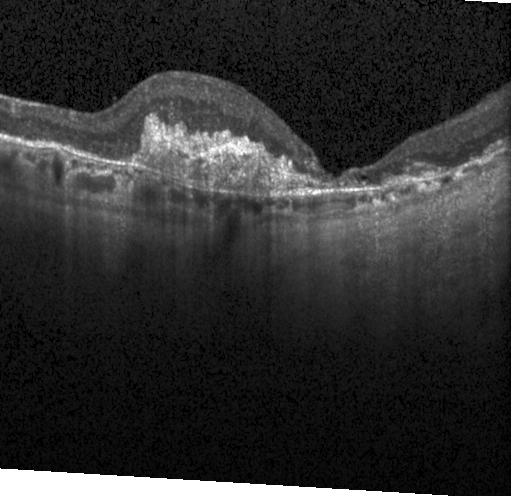

OCT finding: choroidal neovascularization (CNV).